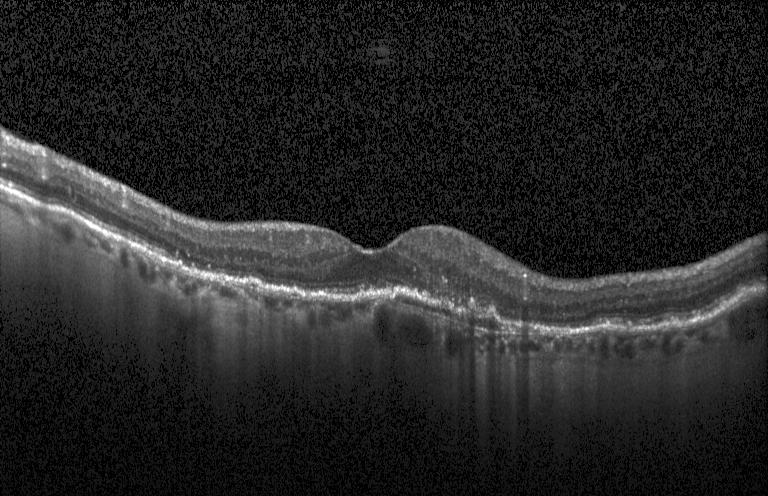
The scan shows a choroidal neovascular membrane.